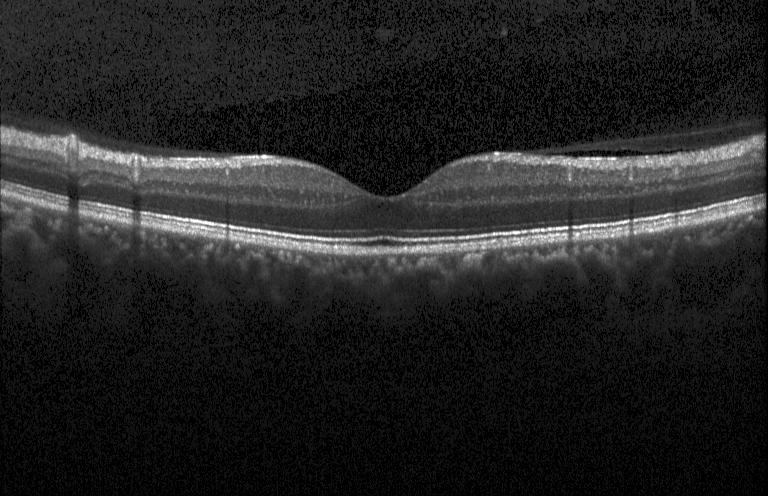

Optical coherence tomography B-scan. Diagnosis: neither choroidal neovascularization, diabetic macular edema, nor drusen.